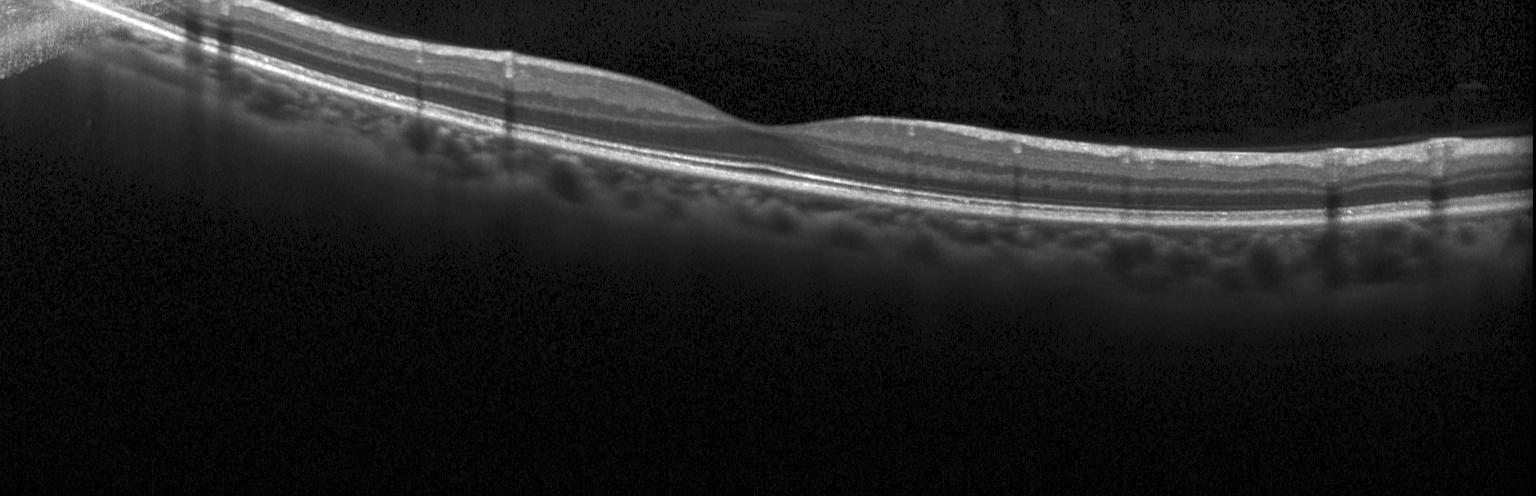

Fovea-centered; SD-OCT; retinal OCT cross-section; Heidelberg Spectralis — Diagnosis: no CNV, no DME, and no drusen.